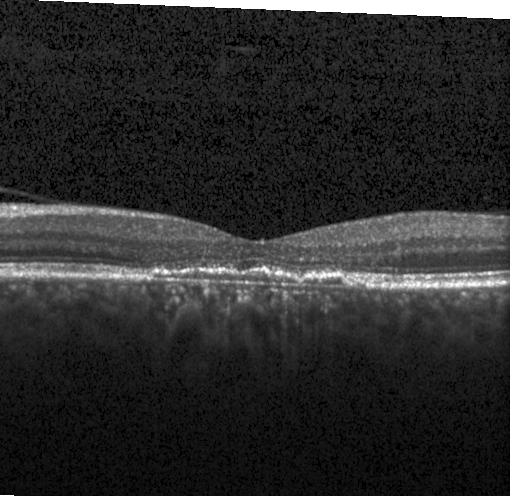

Spectral-domain OCT. Heidelberg Spectralis OCT system. Macular scan. Optical coherence tomography scan
The scan shows a choroidal neovascular membrane.